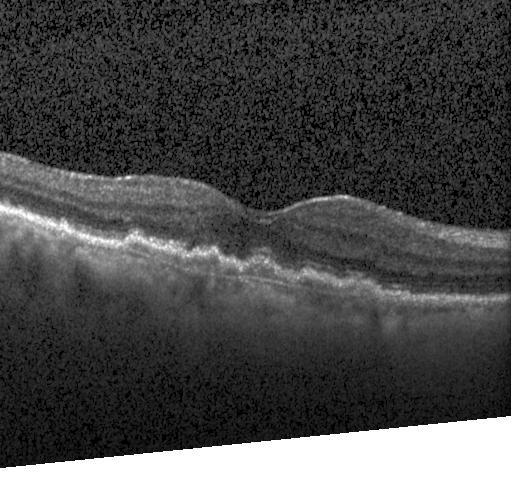 Optical coherence tomography B-scan
Finding: CNV.